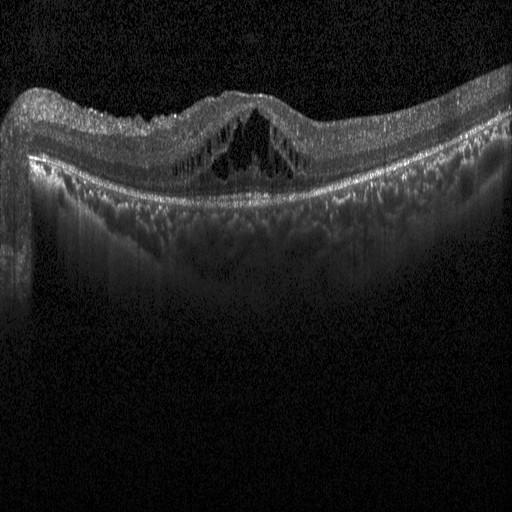

This B-scan demonstrates DME.